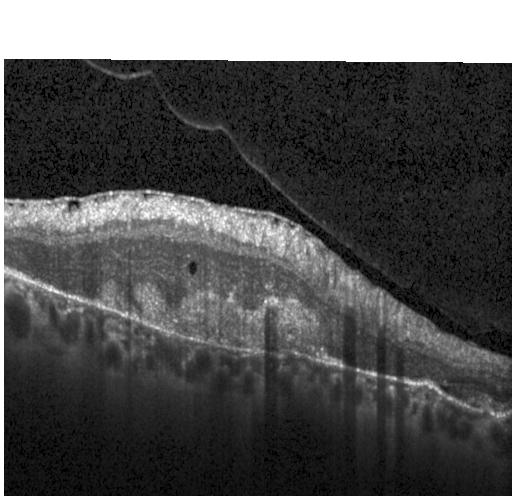

OCT B-scan showing CNV.